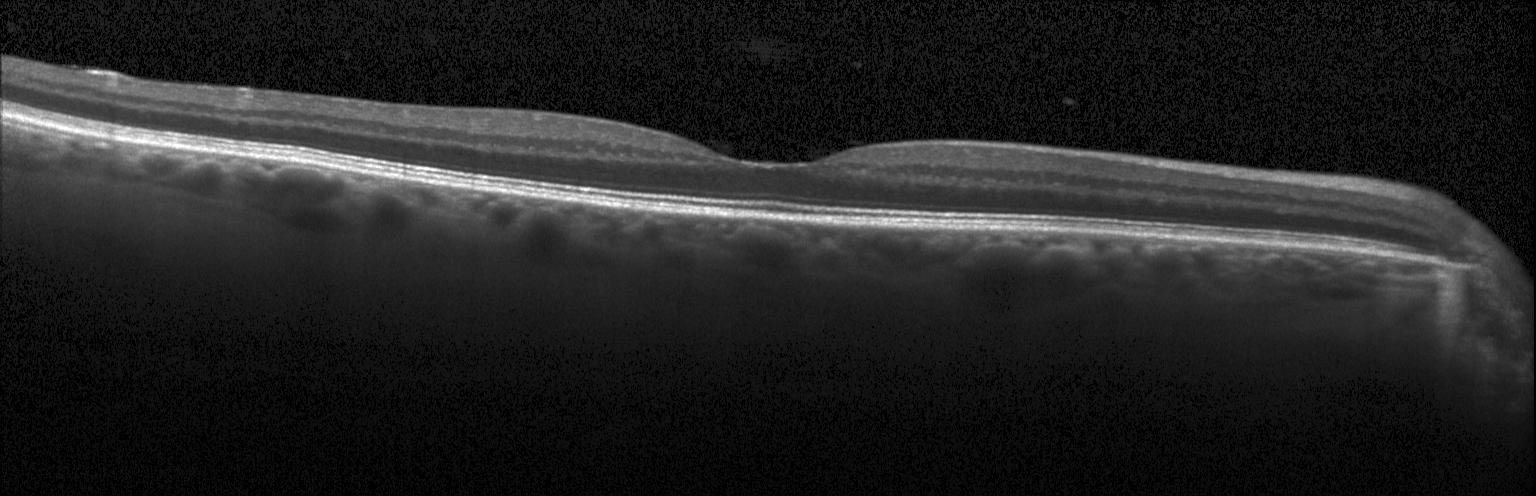 Heidelberg Spectralis OCT system, OCT B-scan. Diagnosis: no CNV, no DME, and no drusen.